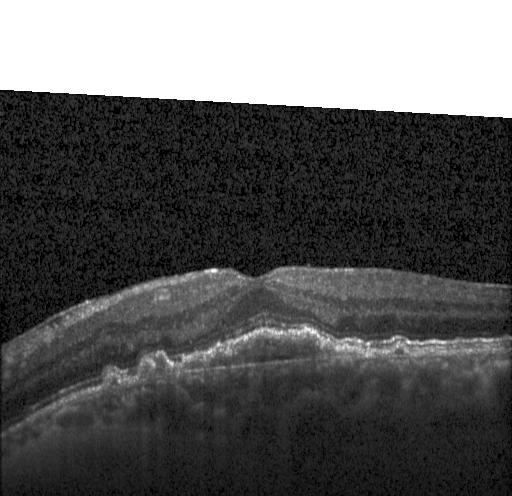 Dx: CNV.